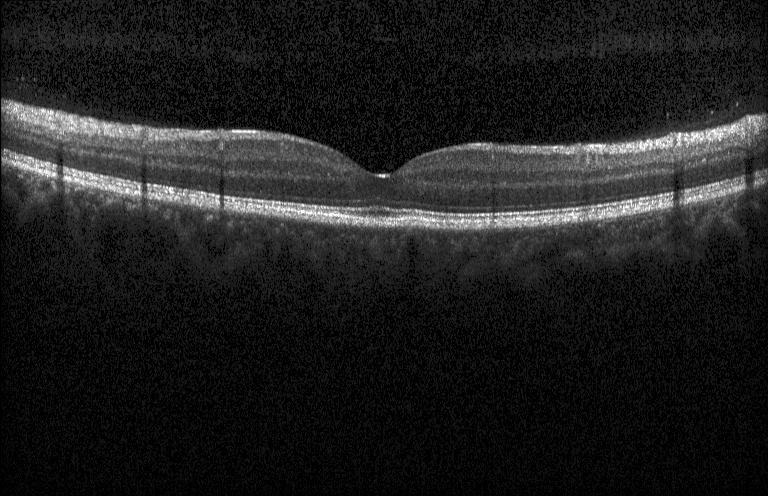
Spectral-domain OCT B-scan: neither choroidal neovascularization, diabetic macular edema, nor drusen.